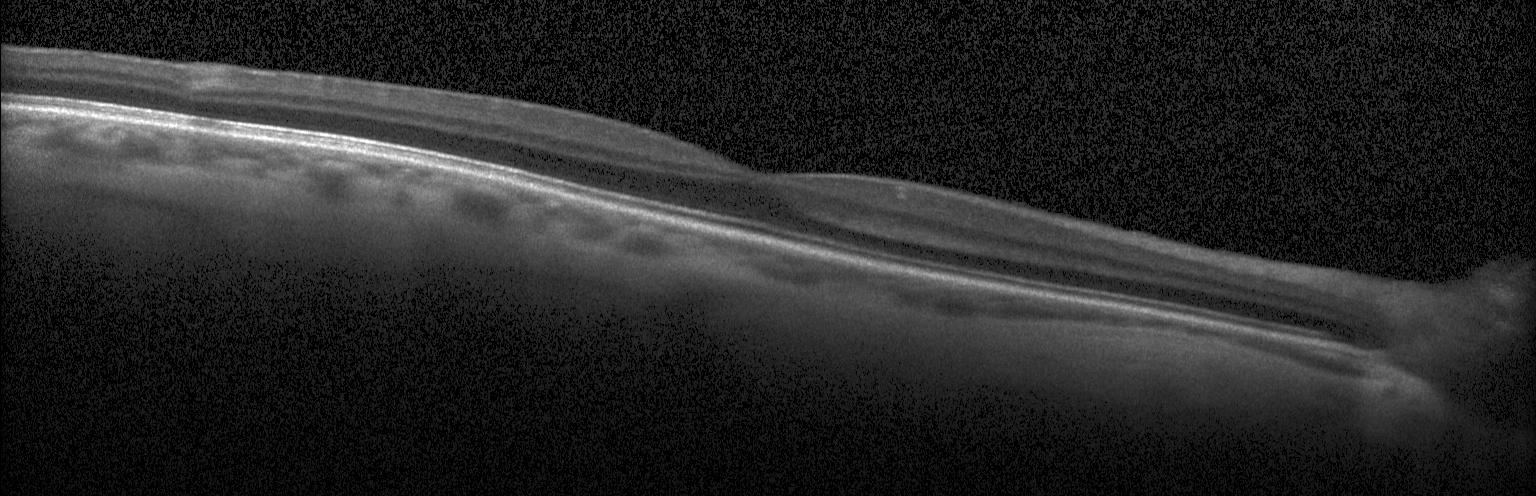

Instrument: Heidelberg Spectralis; spectral-domain OCT; optical coherence tomography scan
Dx: no evidence of CNV, DME, or drusen.